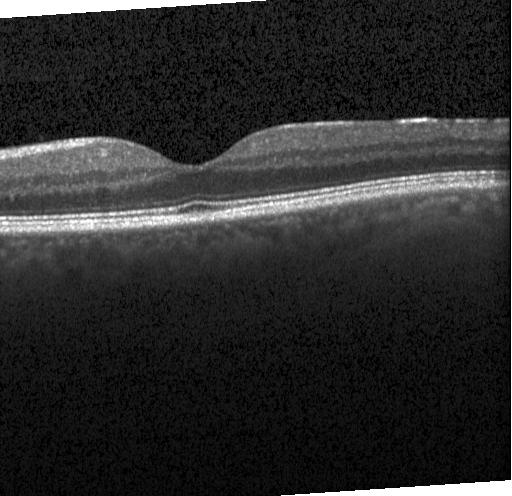 Optical coherence tomography B-scan; centered on the fovea.
OCT finding: no CNV, DME, or drusen.